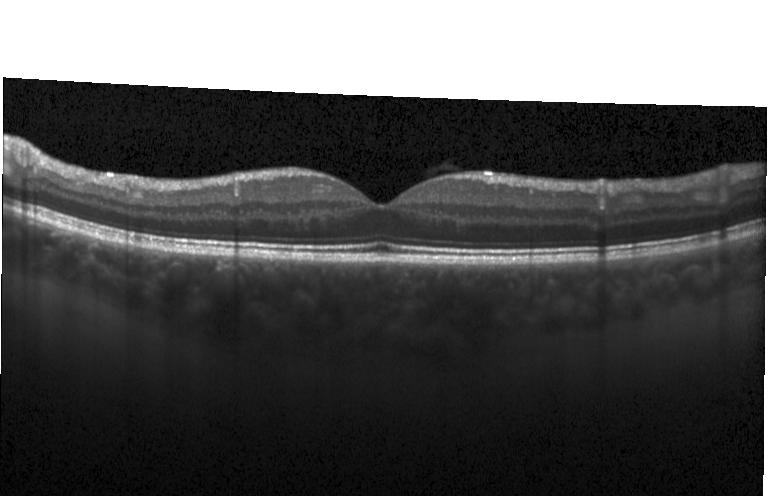 Heidelberg Spectralis, optical coherence tomography B-scan, centered on the fovea
No choroidal neovascularization, diabetic macular edema, or drusen.